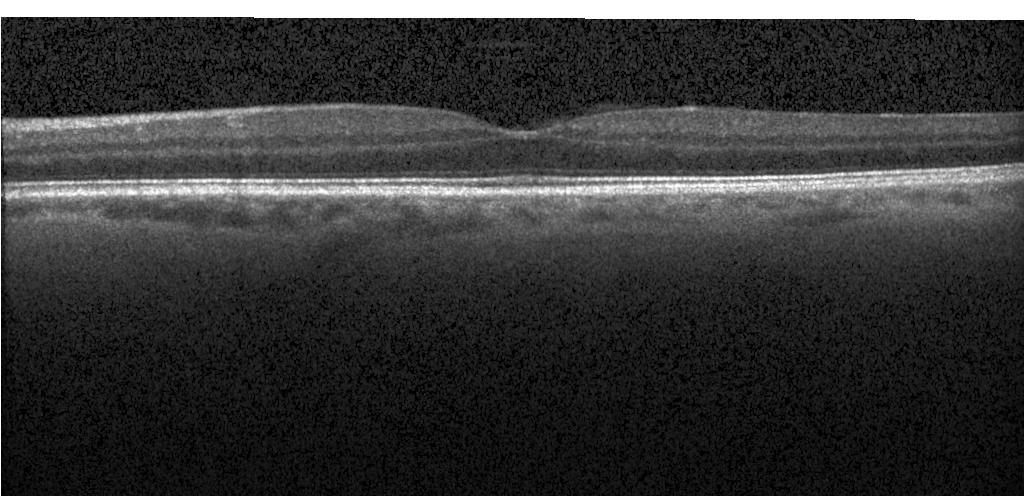

Diagnosis: no choroidal neovascularization, diabetic macular edema, or drusen.